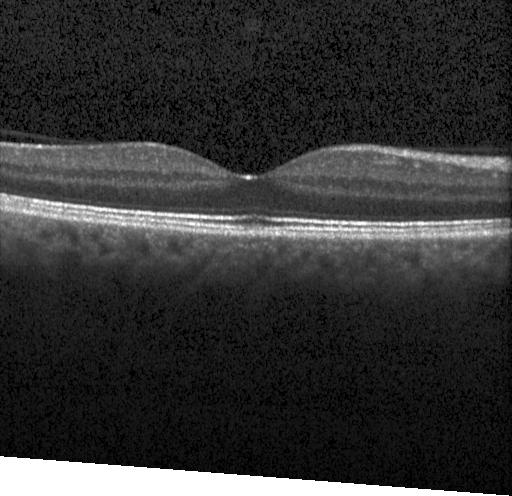
Macular OCT demonstrating no choroidal neovascularization, diabetic macular edema, or drusen.